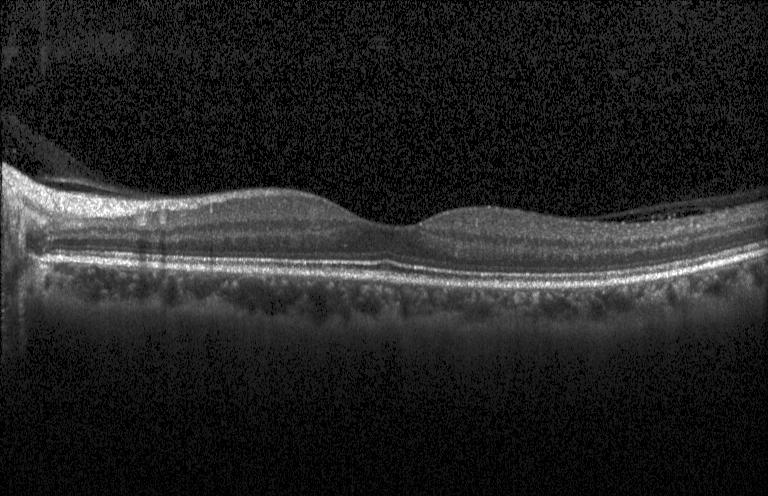

This B-scan demonstrates no choroidal neovascularization, diabetic macular edema, or drusen.